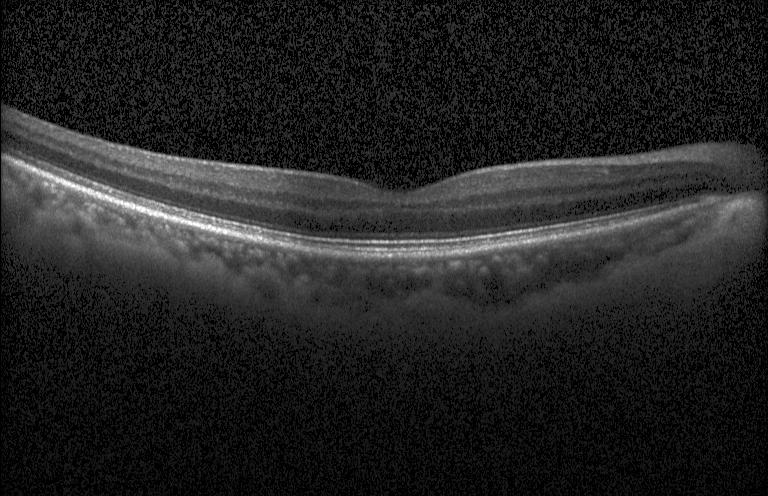

Heidelberg Spectralis; OCT line scan — Finding: no CNV, DME, or drusen.